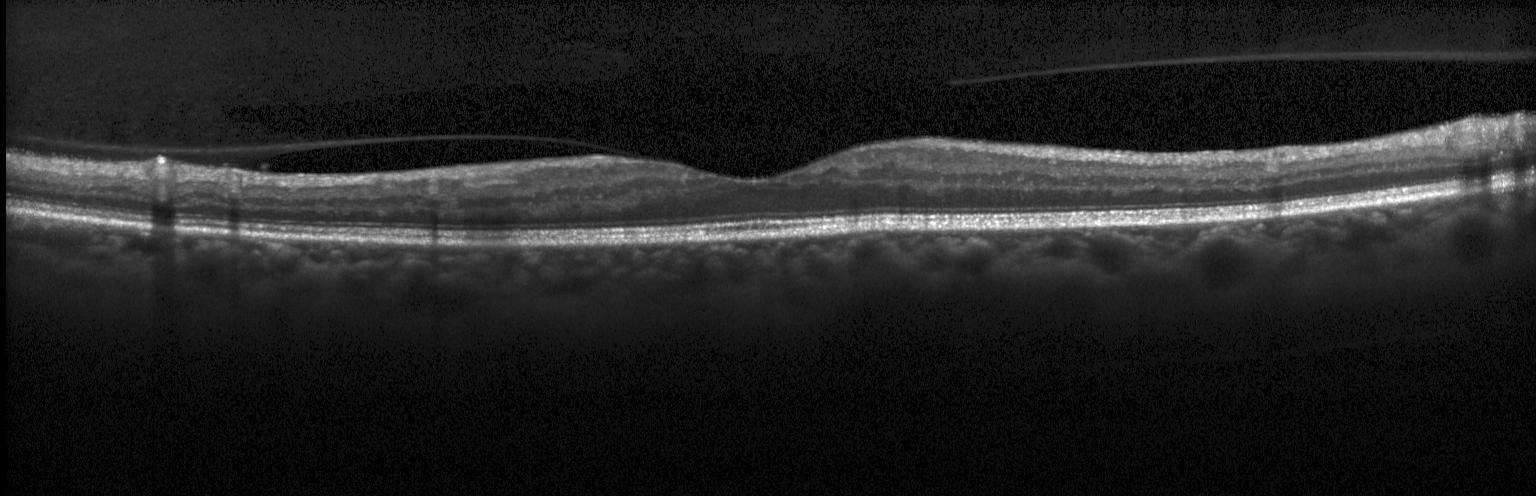
Dx: no choroidal neovascularization, no diabetic macular edema, and no drusen.